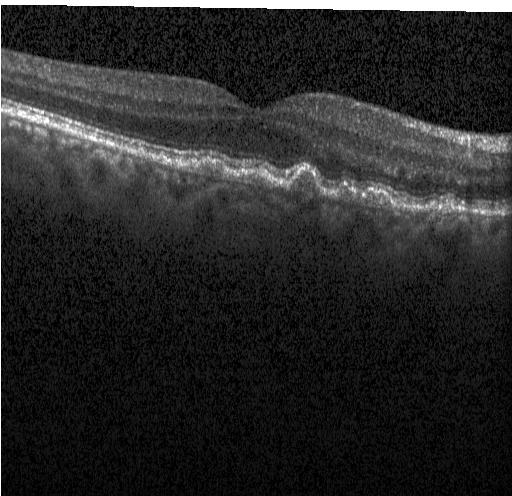

Retinal OCT B-scan. Multiple drusen.